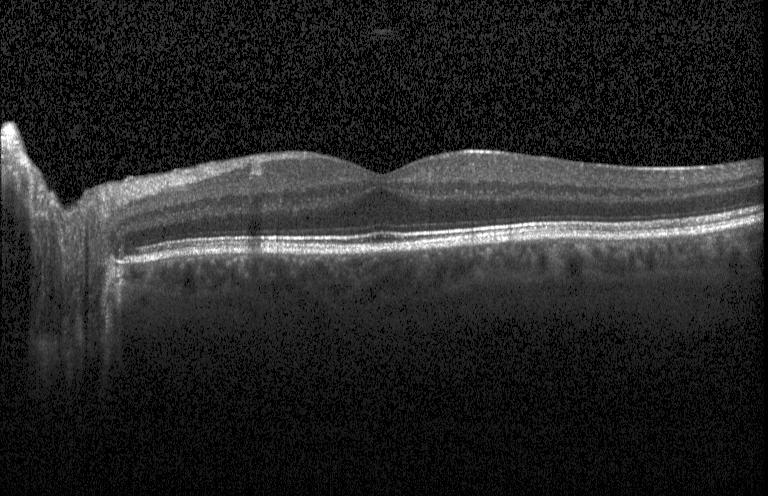
Optical coherence tomography B-scan. No choroidal neovascularization, no diabetic macular edema, and no drusen.